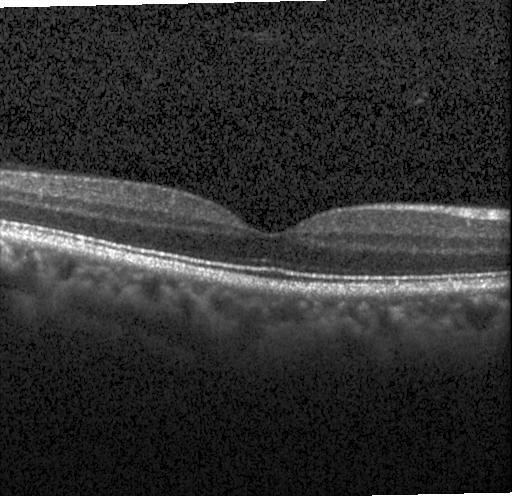

Finding: neither choroidal neovascularization, diabetic macular edema, nor drusen.